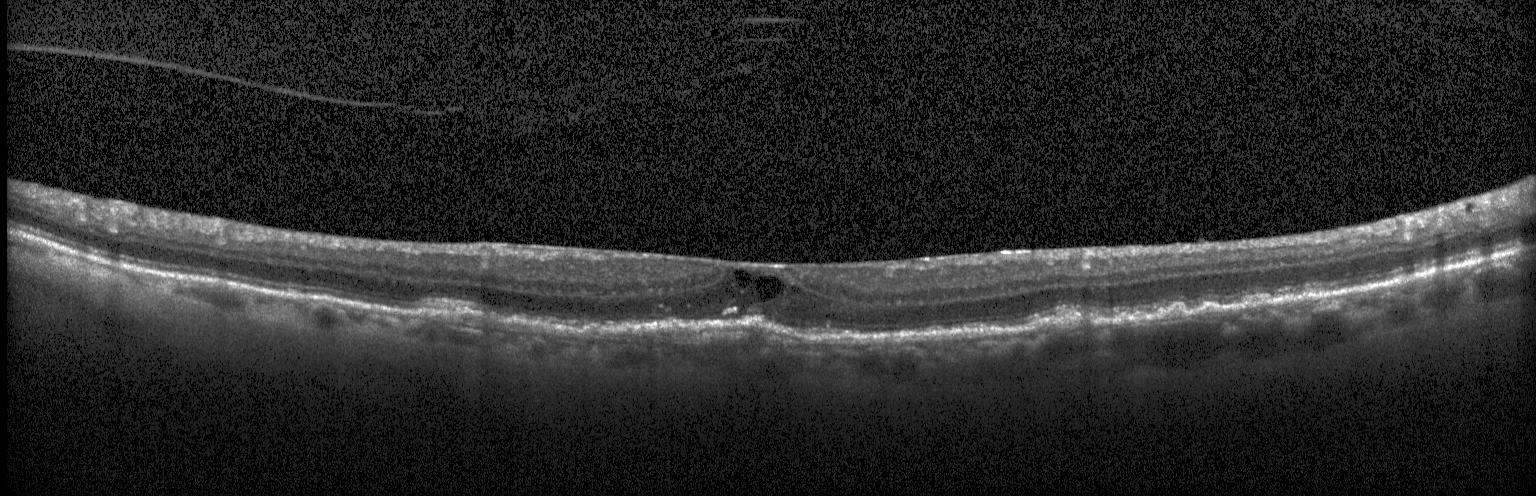 OCT line scan
Assessment: a choroidal neovascular membrane.